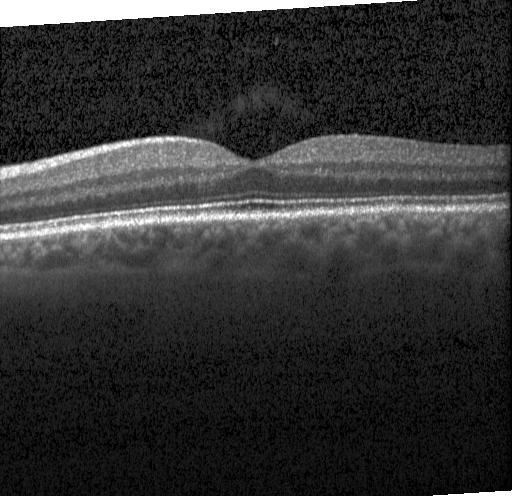

Finding: neither CNV, DME, nor drusen.